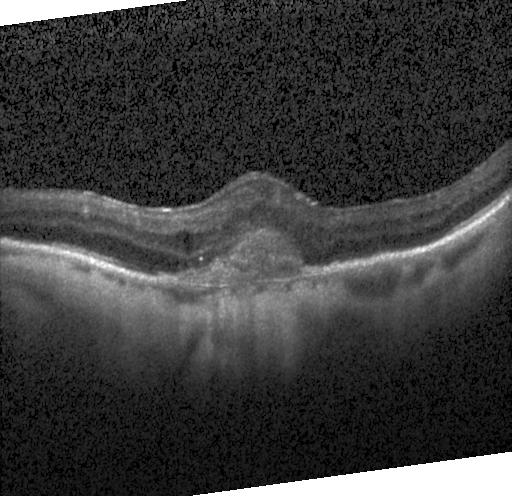

Instrument: Heidelberg Spectralis · SD-OCT · optical coherence tomography scan. OCT finding: a choroidal neovascular membrane.